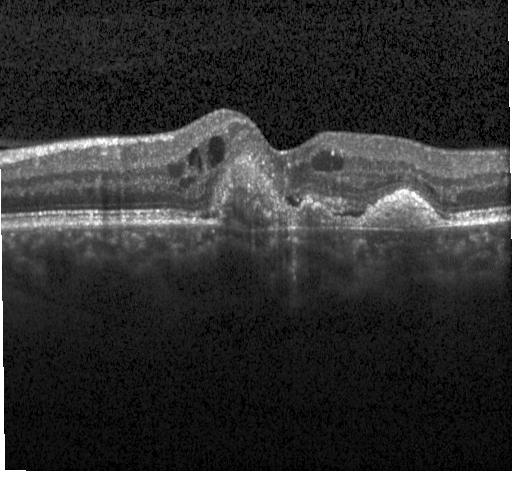
Retinal OCT cross-section showing choroidal neovascularization.